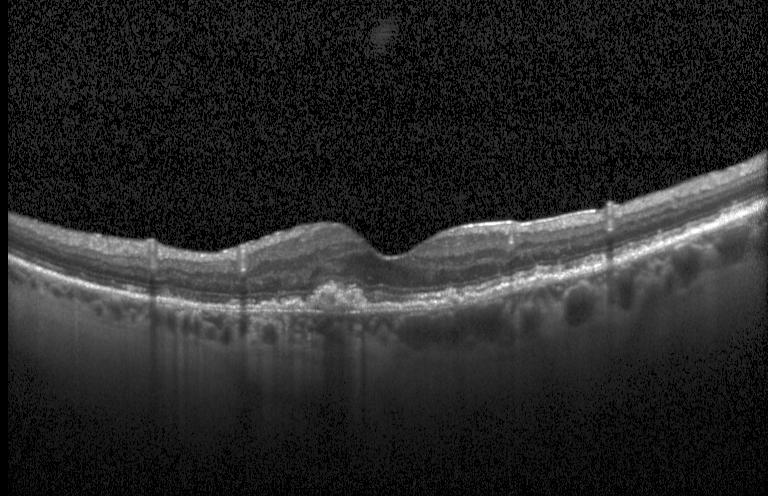

Through the macula. Instrument: Heidelberg Spectralis. Optical coherence tomography B-scan — The scan shows a choroidal neovascular membrane.